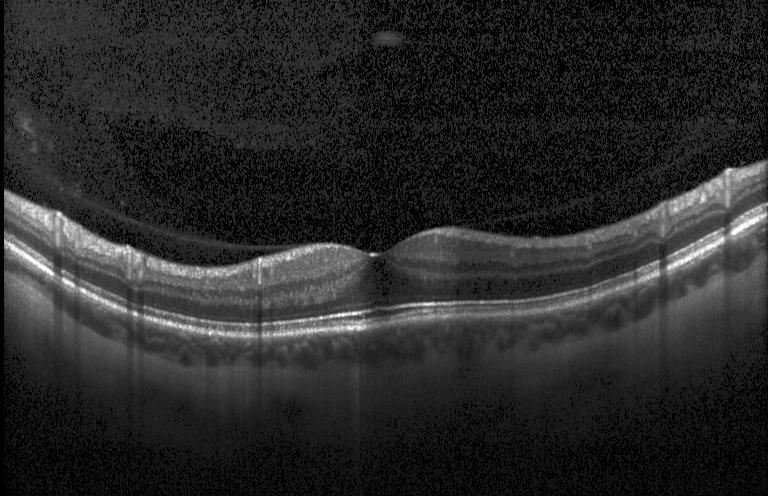 OCT line scan; through the macula; spectral-domain OCT — Diagnosis: no choroidal neovascularization, no diabetic macular edema, and no drusen.